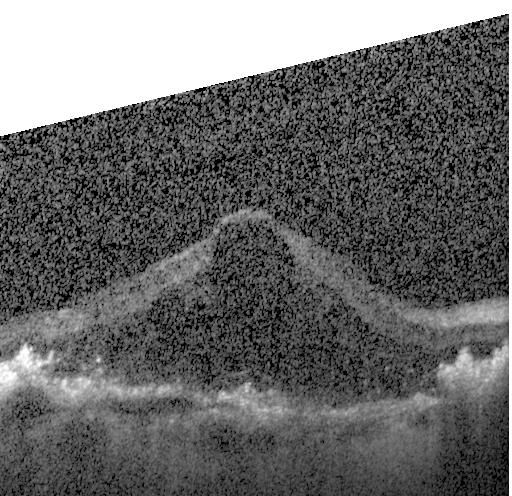 Fovea-centered; spectral-domain optical coherence tomography; optical coherence tomography B-scan
A choroidal neovascular membrane.